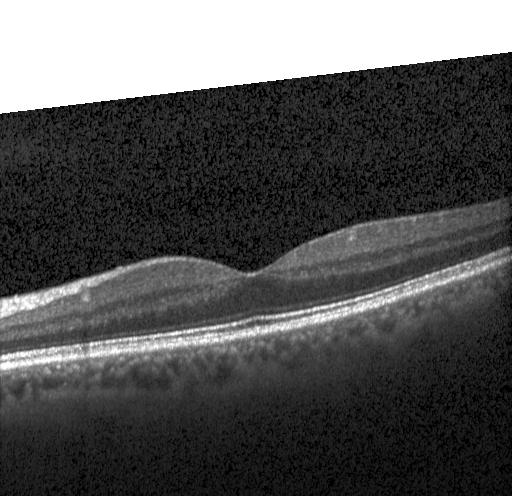

The scan shows neither choroidal neovascularization, diabetic macular edema, nor drusen.